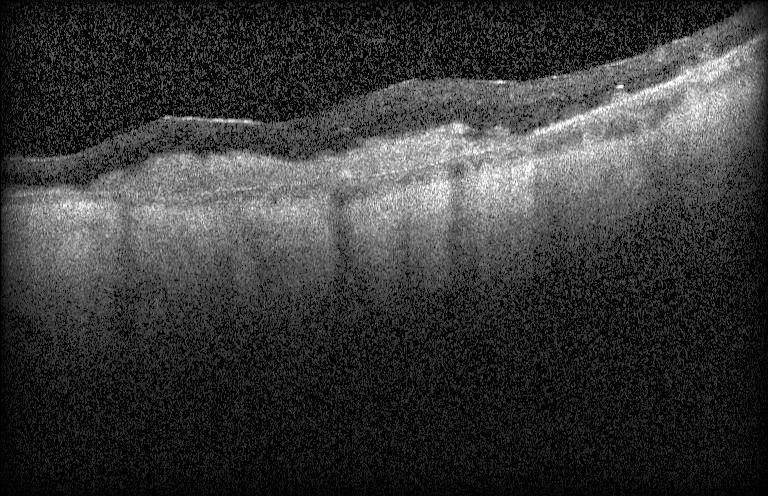

Impression: a choroidal neovascular membrane.